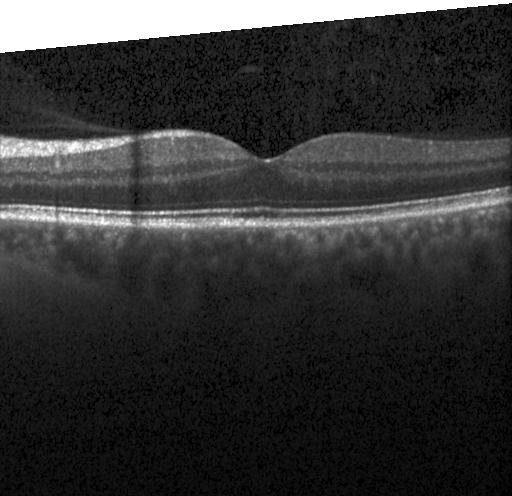

Heidelberg Spectralis OCT system. SD-OCT. Horizontal scan through the fovea. Optical coherence tomography scan — The scan shows no evidence of CNV, DME, or drusen.